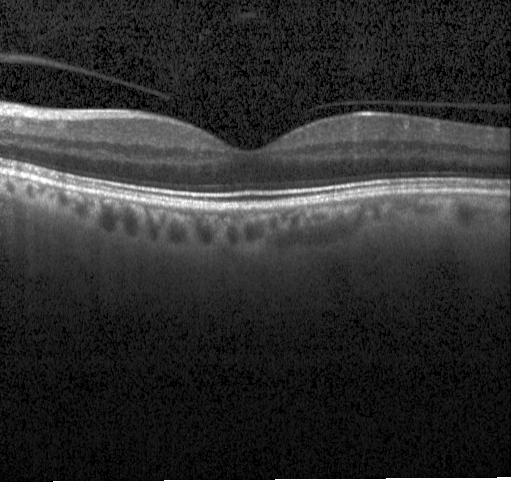

Spectral-domain optical coherence tomography. OCT B-scan. Acquired on a Heidelberg Spectralis. Centered on the fovea — Impression: no CNV, no DME, and no drusen.